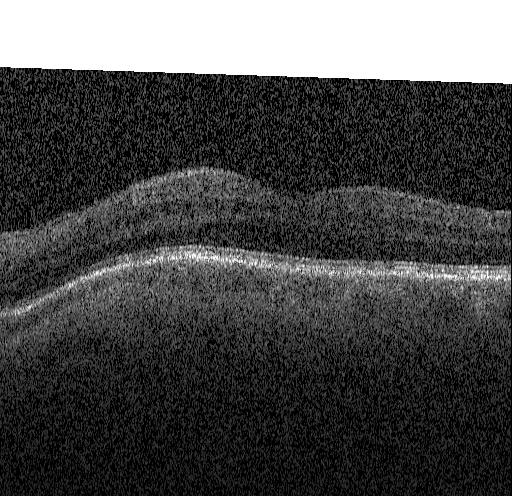
OCT B-scan. This B-scan demonstrates no choroidal neovascularization, no diabetic macular edema, and no drusen.